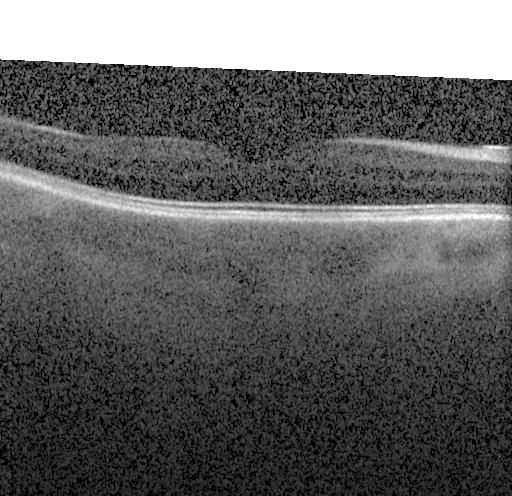 OCT line scan · spectral-domain optical coherence tomography · macular scan.
Dx: no CNV, DME, or drusen.